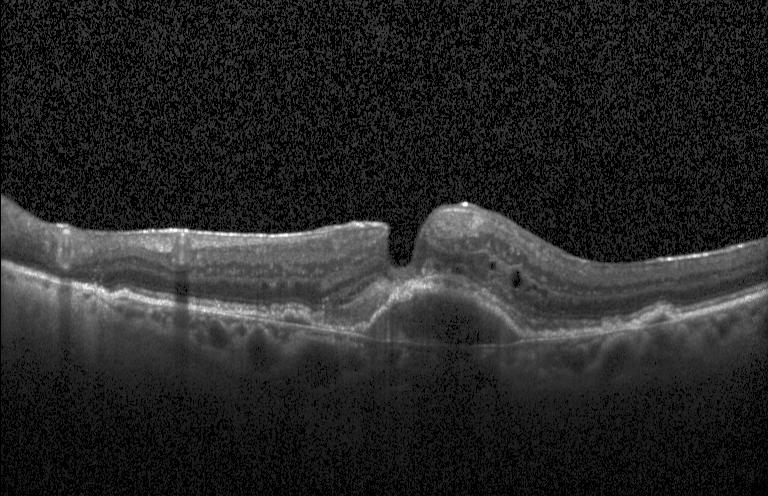 OCT scan showing CNV.